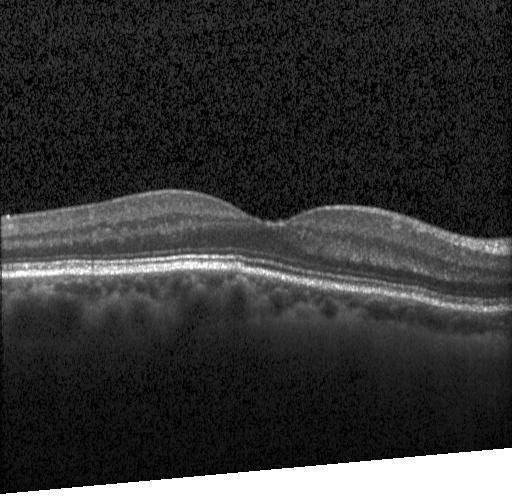

Acquired on a Heidelberg Spectralis. SD-OCT. Retinal OCT cross-section.
Diagnosis: no CNV, DME, or drusen.